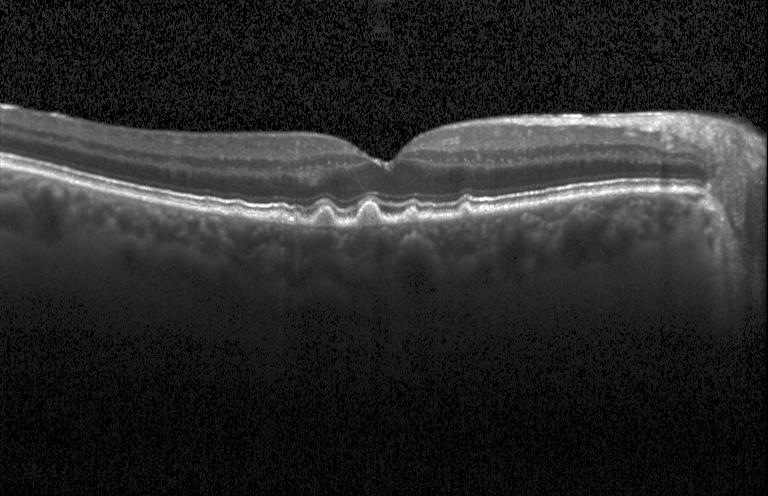
Dx: multiple drusen.